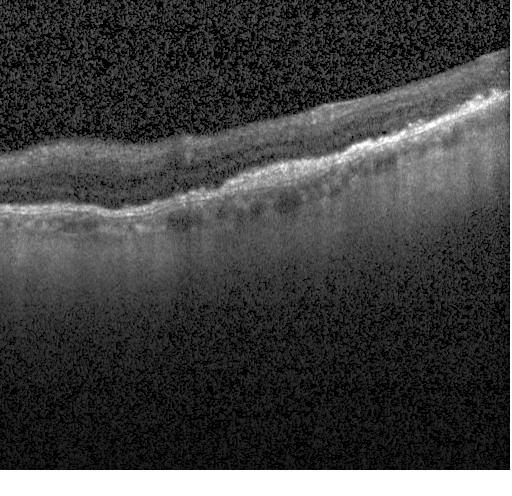

Centered on the fovea; retinal OCT B-scan.
Dx: a choroidal neovascular membrane.